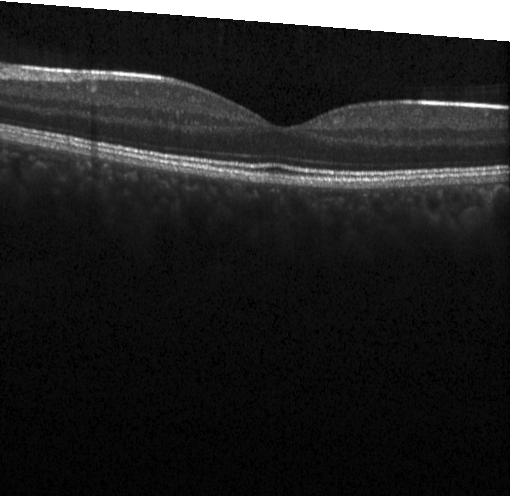

Heidelberg Spectralis OCT system. SD-OCT. Through the macula. OCT B-scan. OCT finding: neither choroidal neovascularization, diabetic macular edema, nor drusen.